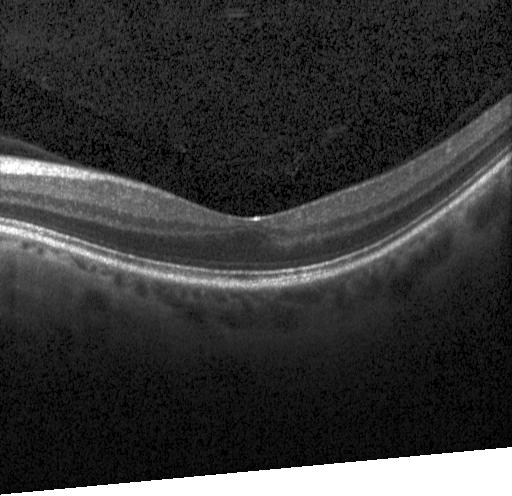 Macular OCT demonstrating no CNV, no DME, and no drusen.